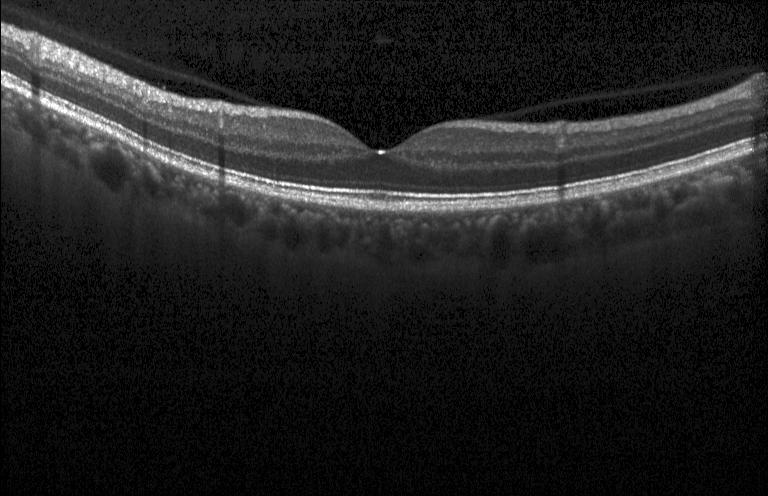
Spectral-domain OCT. OCT line scan. Through the macula.
Dx: no evidence of CNV, DME, or drusen.